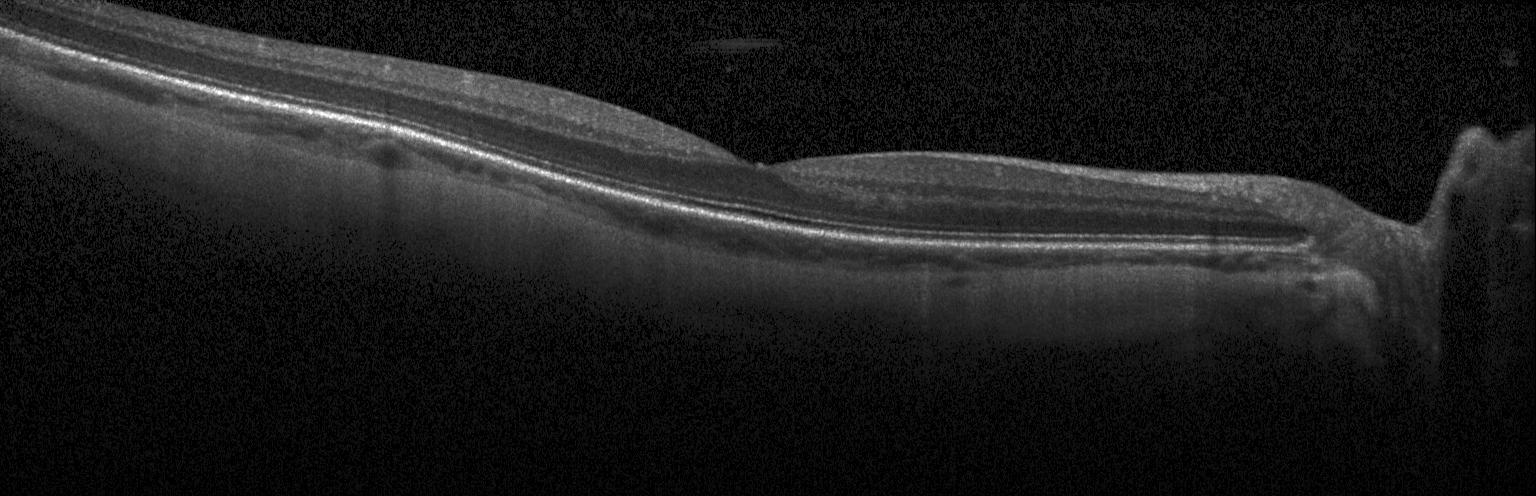
Acquired on a Heidelberg Spectralis; optical coherence tomography B-scan; spectral-domain optical coherence tomography; macular scan. Dx: no evidence of CNV, DME, or drusen.